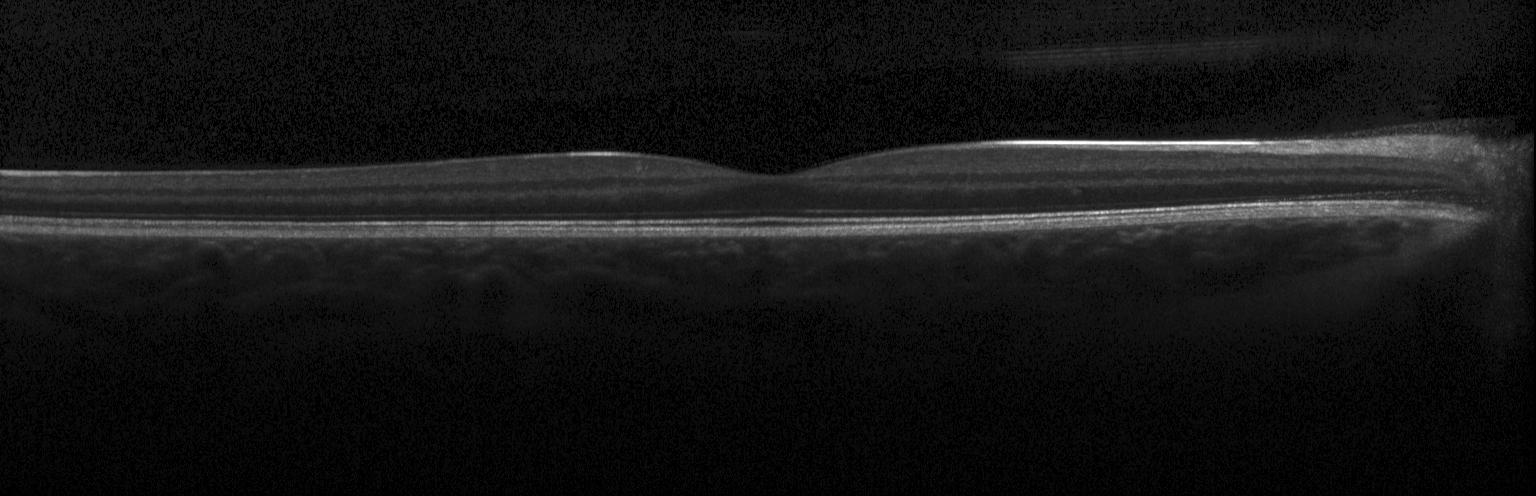
This B-scan demonstrates no CNV, no DME, and no drusen.